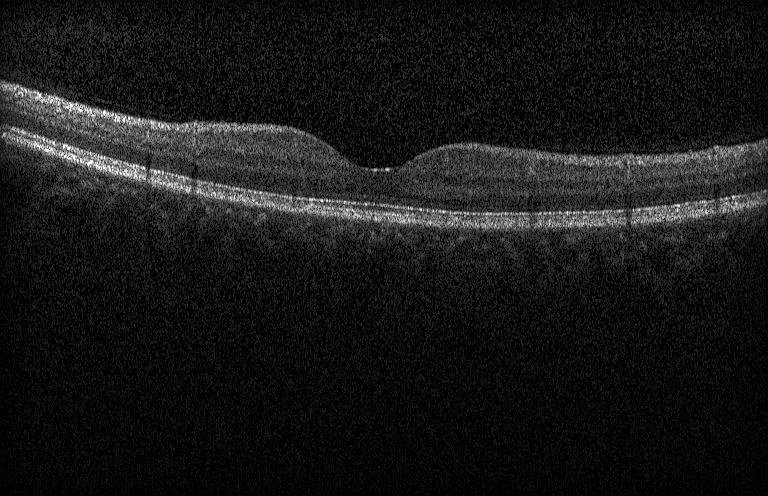
OCT line scan.
Impression: neither CNV, DME, nor drusen.